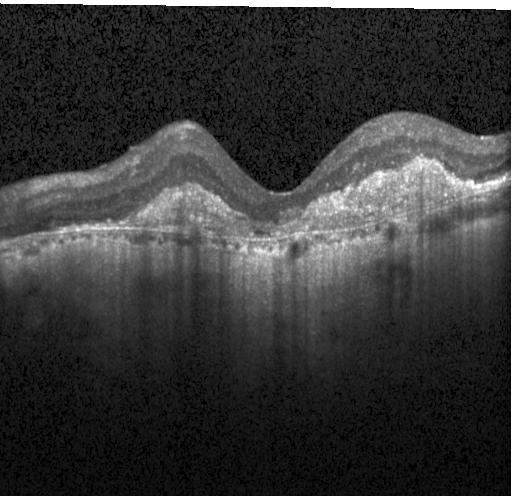 Dx: a choroidal neovascular membrane.